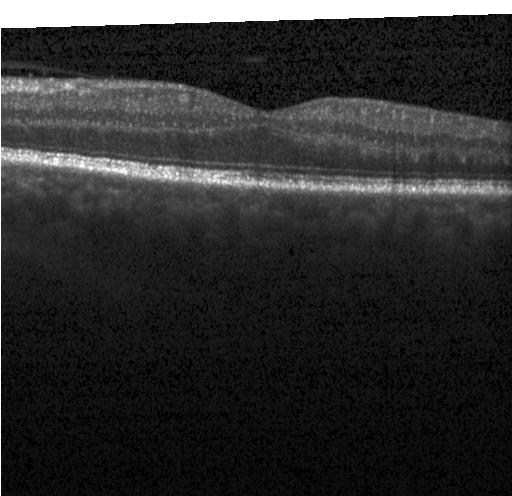 OCT B-scan, centered on the fovea, SD-OCT.
Impression: no choroidal neovascularization, diabetic macular edema, or drusen.